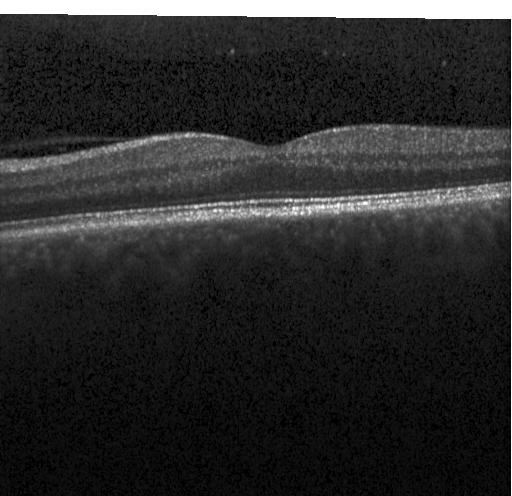 Optical coherence tomography B-scan; Heidelberg Spectralis
OCT finding: no CNV, no DME, and no drusen.